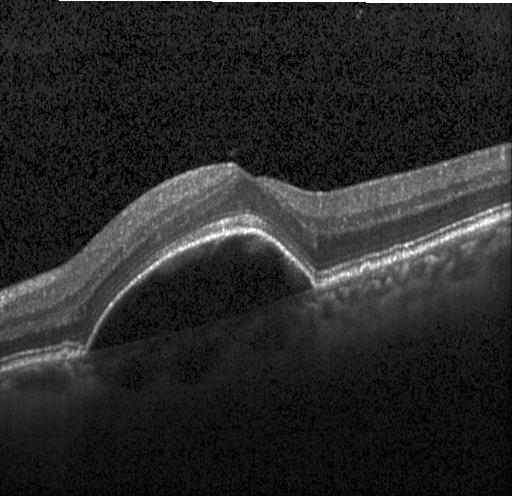

OCT finding: choroidal neovascularization (CNV).